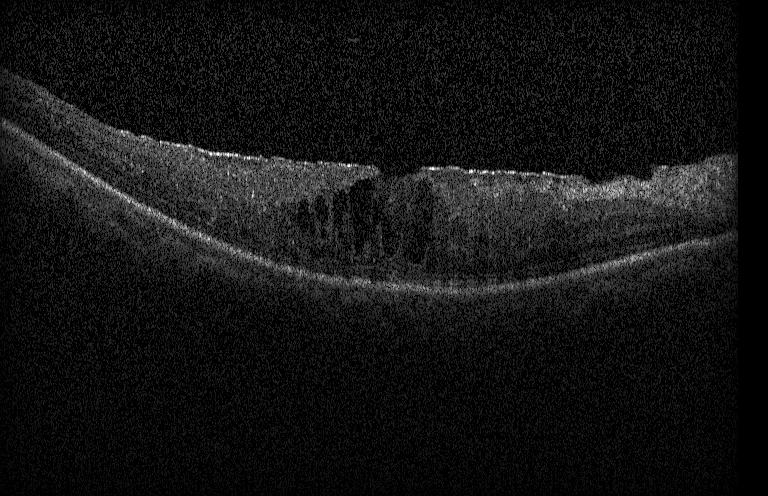
Diabetic macular edema.